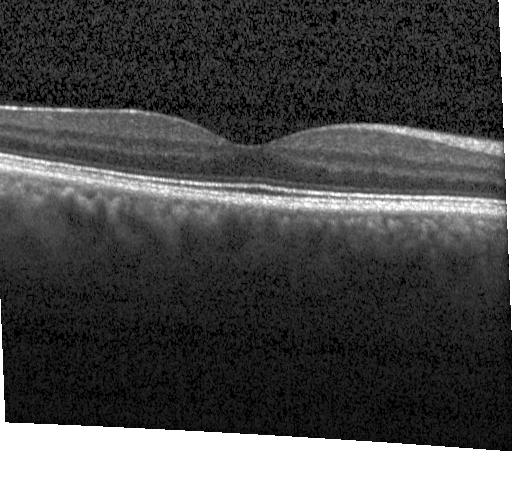 Spectral-domain optical coherence tomography, Heidelberg Spectralis OCT system, through the macula, optical coherence tomography B-scan. The scan shows no evidence of CNV, DME, or drusen.